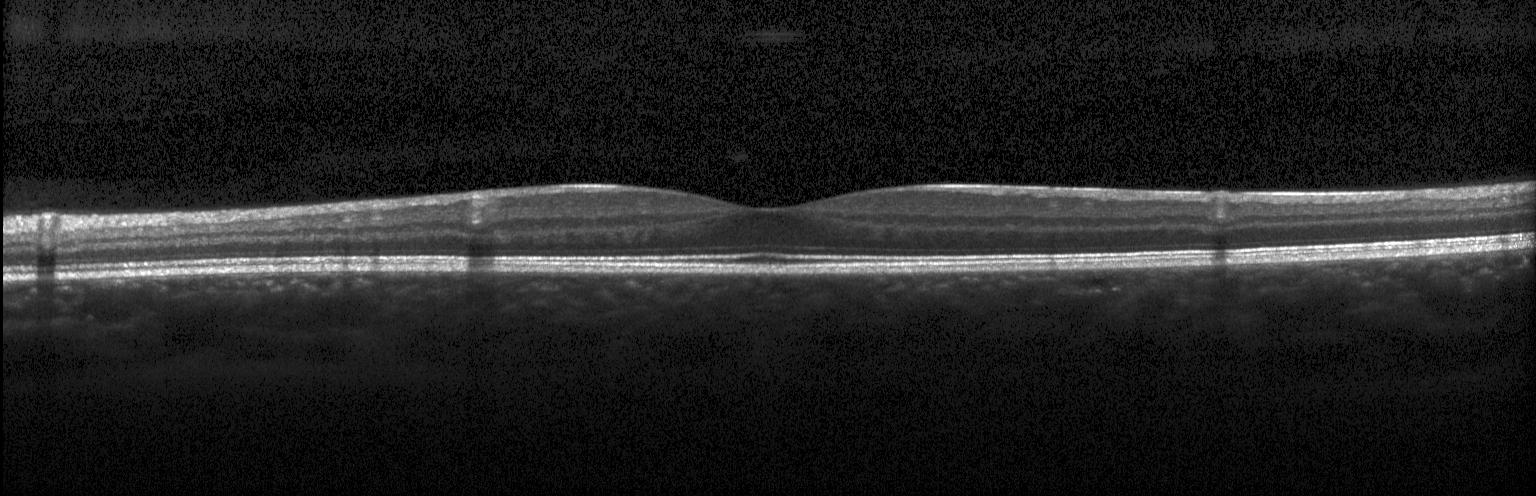

Assessment: neither choroidal neovascularization, diabetic macular edema, nor drusen.